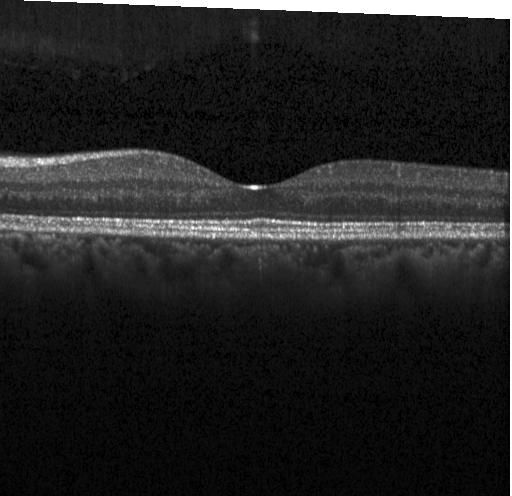

OCT B-scan. Horizontal scan through the fovea
Impression: neither CNV, DME, nor drusen.